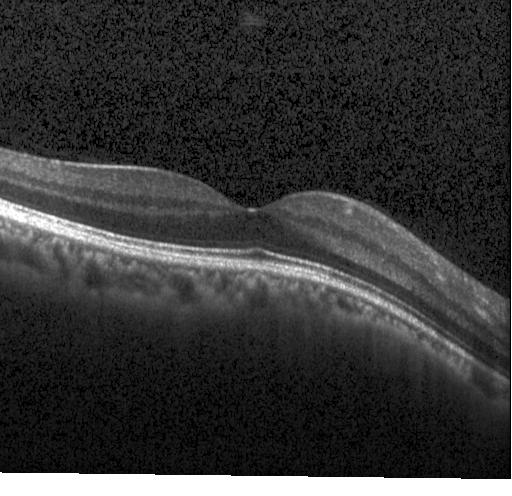 Impression: no choroidal neovascularization, diabetic macular edema, or drusen.